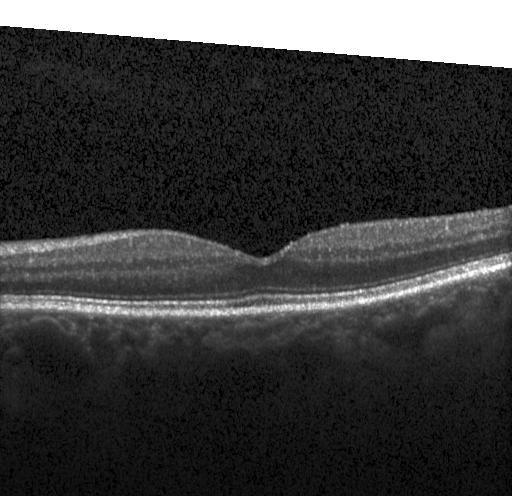 Retinal OCT B-scan — Diagnosis: neither choroidal neovascularization, diabetic macular edema, nor drusen.